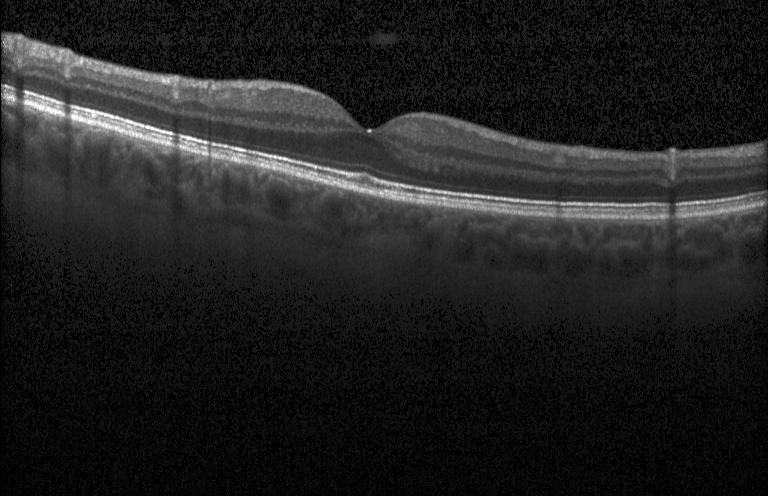

Macular scan, optical coherence tomography B-scan, acquired on a Heidelberg Spectralis, SD-OCT
Diagnosis: no choroidal neovascularization, no diabetic macular edema, and no drusen.